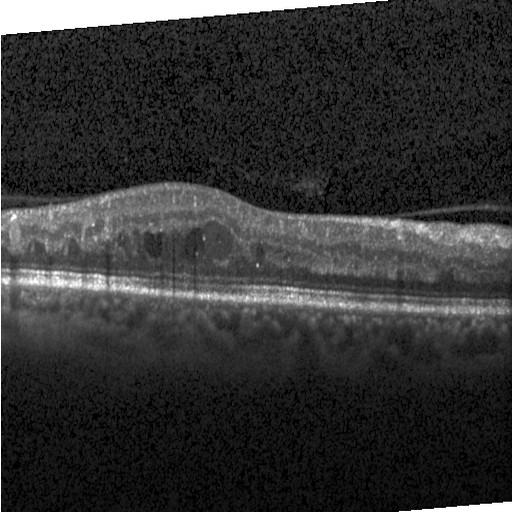

Optical coherence tomography B-scan
OCT finding: diabetic macular edema (DME).